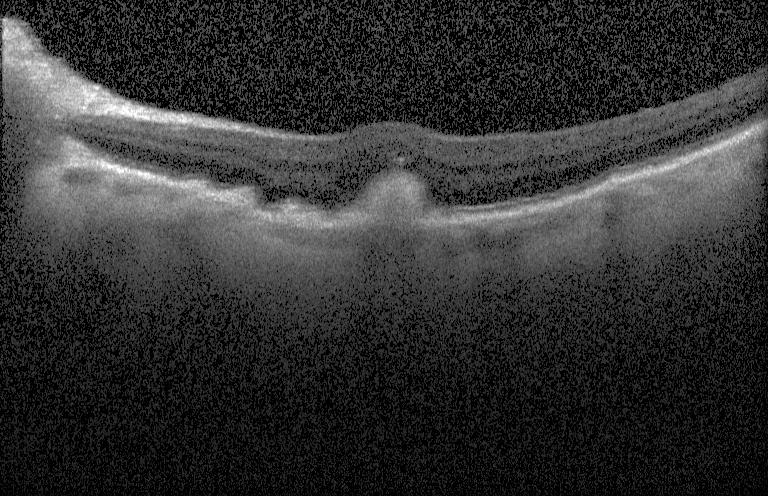
Optical coherence tomography B-scan — OCT finding: sub-RPE drusenoid deposits.